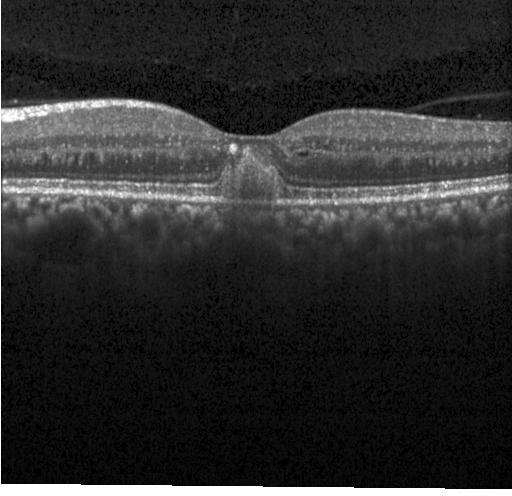 Retinal OCT cross-section, fovea-centered
Dx: a choroidal neovascular membrane.